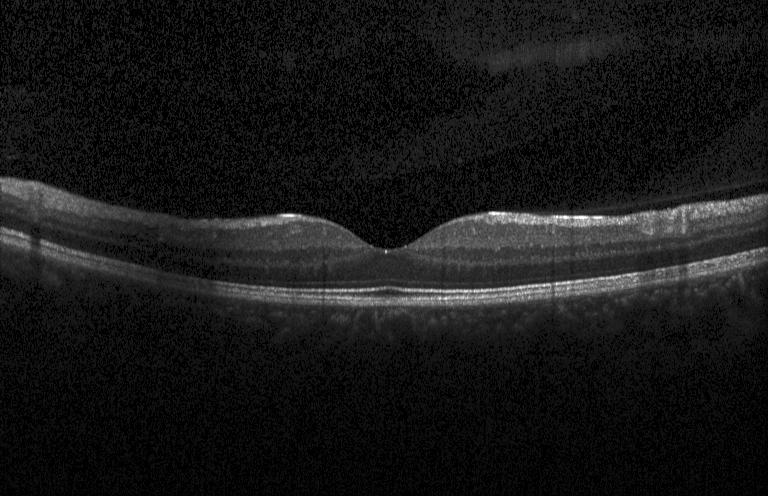

Optical coherence tomography scan — Impression: no evidence of choroidal neovascularization, diabetic macular edema, or drusen.